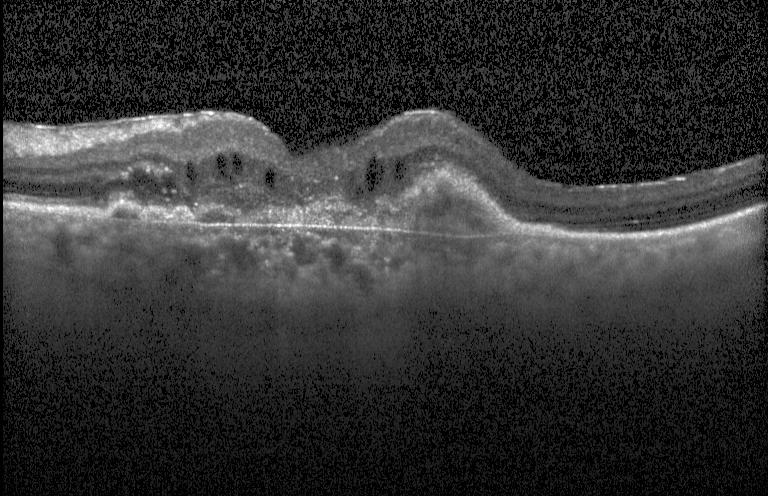
Choroidal neovascularization.